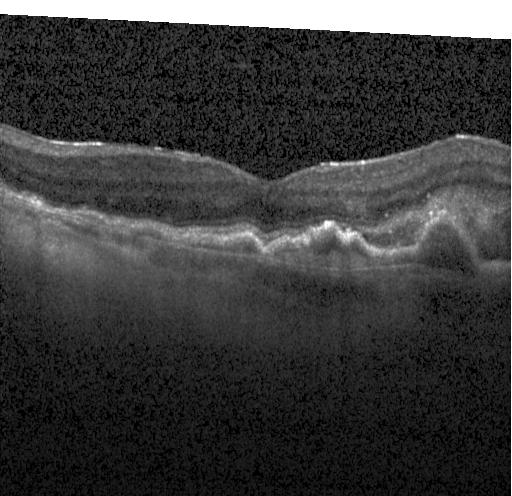 OCT line scan · SD-OCT · Heidelberg Spectralis. Finding: a choroidal neovascular membrane.